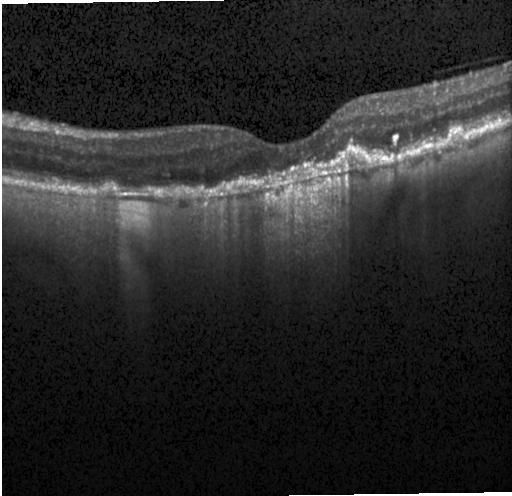
A choroidal neovascular membrane.